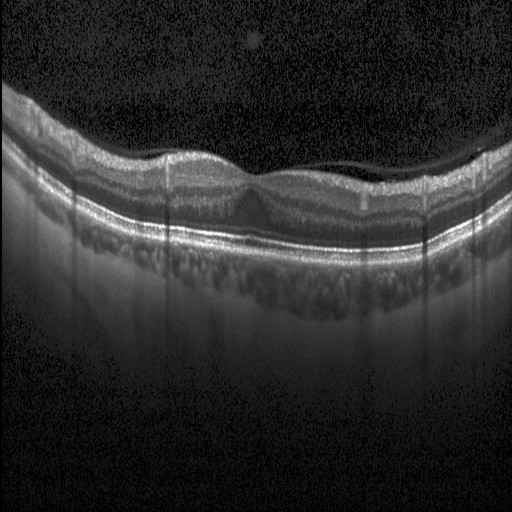
Finding: diabetic macular edema.